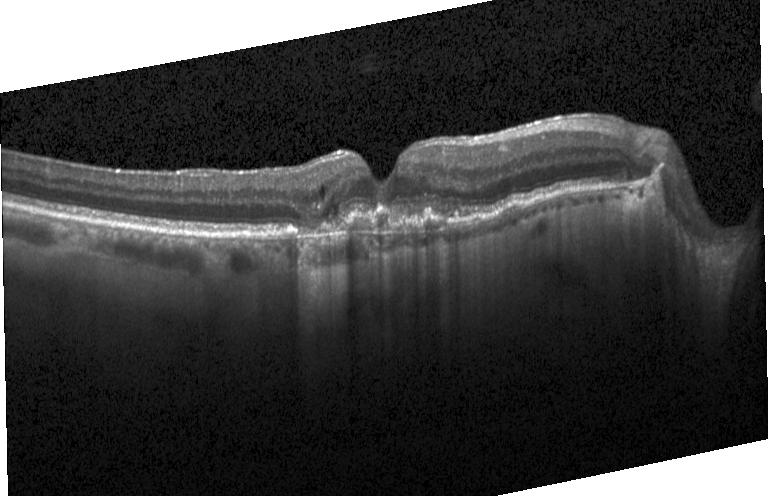

Retinal OCT B-scan, Heidelberg Spectralis, fovea-centered, spectral-domain OCT.
Assessment: choroidal neovascularization (CNV).